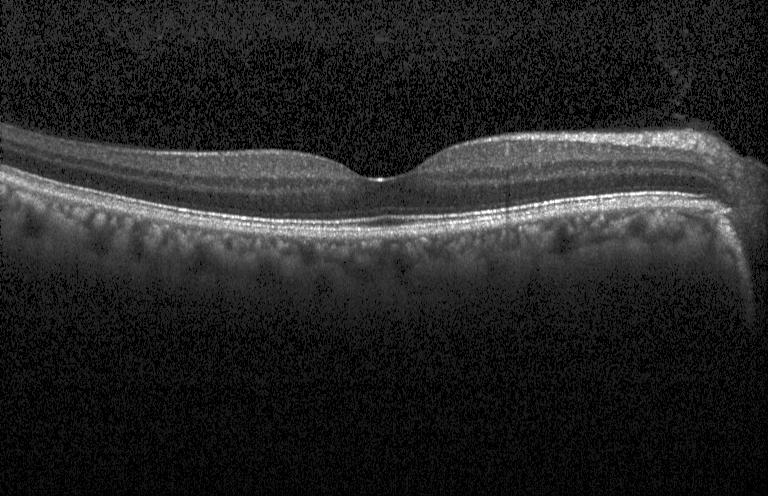 No CNV, DME, or drusen.